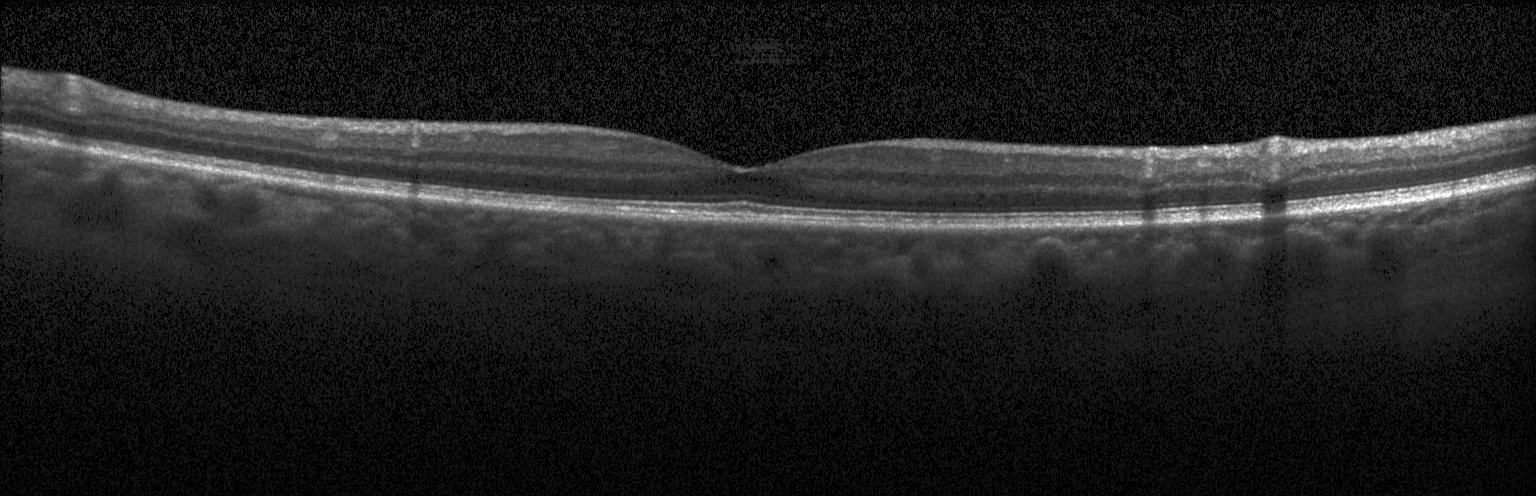

SD-OCT. Centered on the fovea. Optical coherence tomography scan
Impression: no evidence of choroidal neovascularization, diabetic macular edema, or drusen.